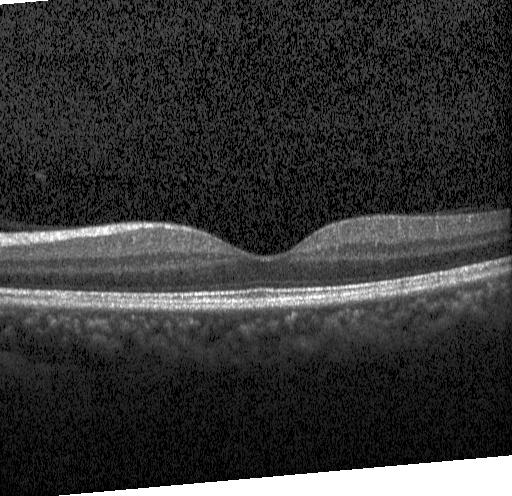
Retinal OCT B-scan.
This B-scan demonstrates no choroidal neovascularization, diabetic macular edema, or drusen.